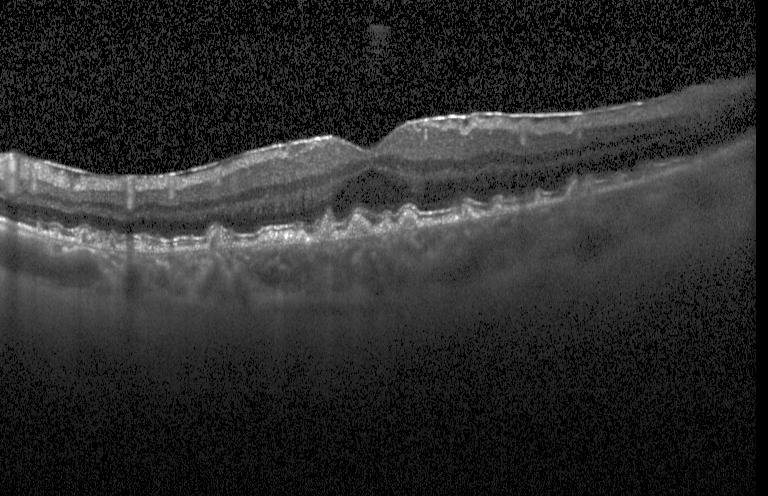

Retinal OCT B-scan
Macular OCT: multiple drusen.